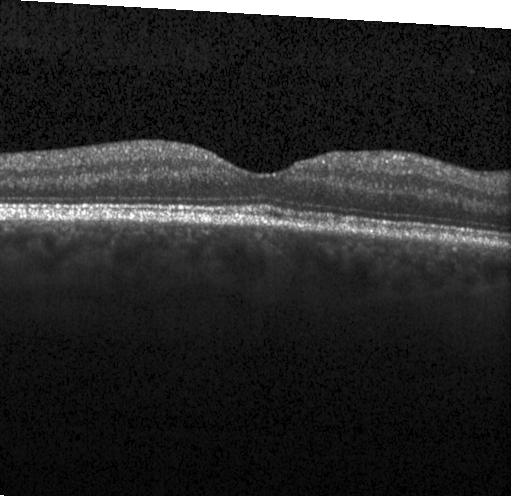 Spectral-domain optical coherence tomography; horizontal scan through the fovea; retinal OCT cross-section
This B-scan demonstrates no choroidal neovascularization, no diabetic macular edema, and no drusen.